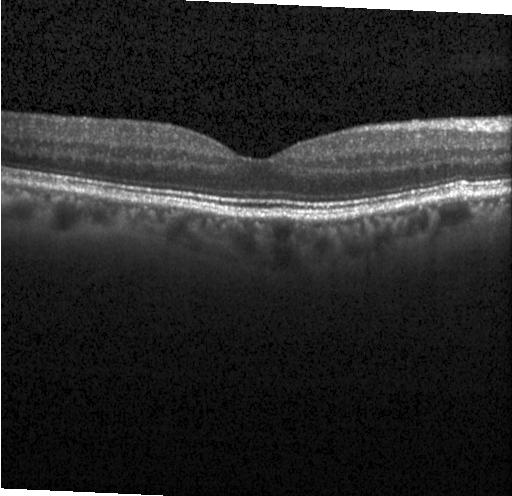

Optical coherence tomography B-scan. The scan shows neither CNV, DME, nor drusen.